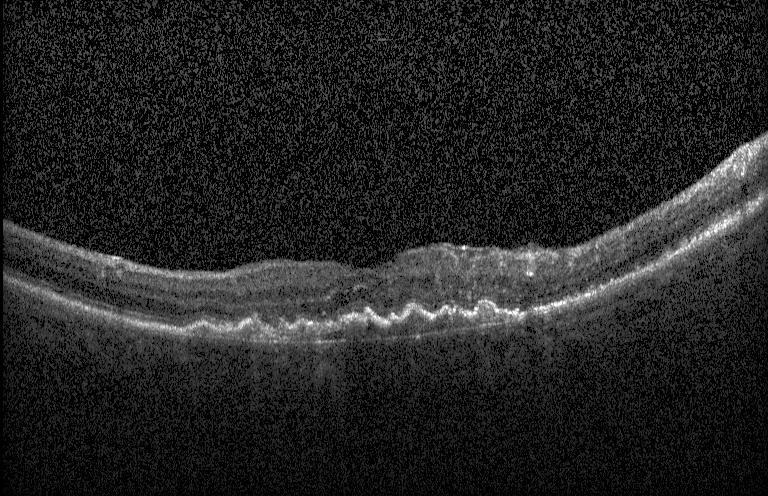 Optical coherence tomography scan
Diagnosis: choroidal neovascularization.